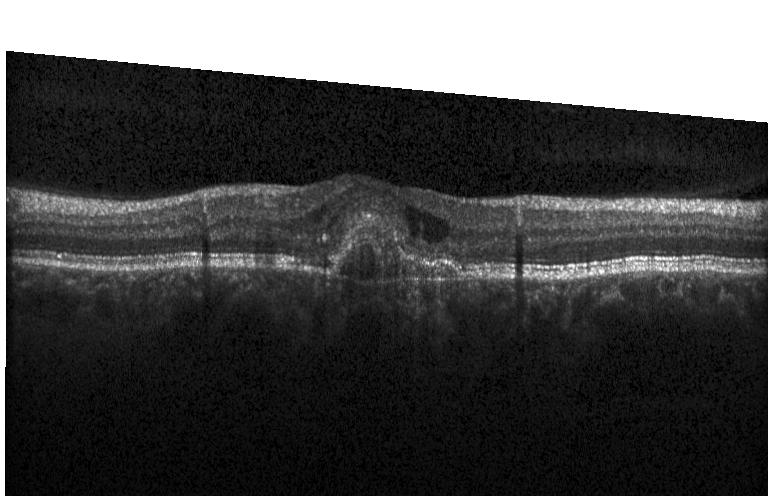

OCT finding: choroidal neovascularization (CNV).